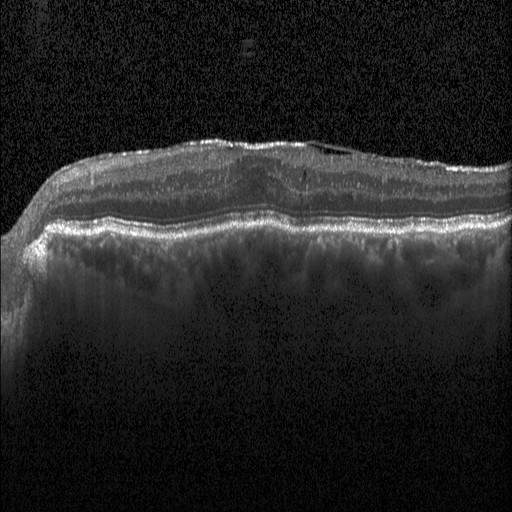

Retinal OCT cross-section showing diabetic macular edema (DME).